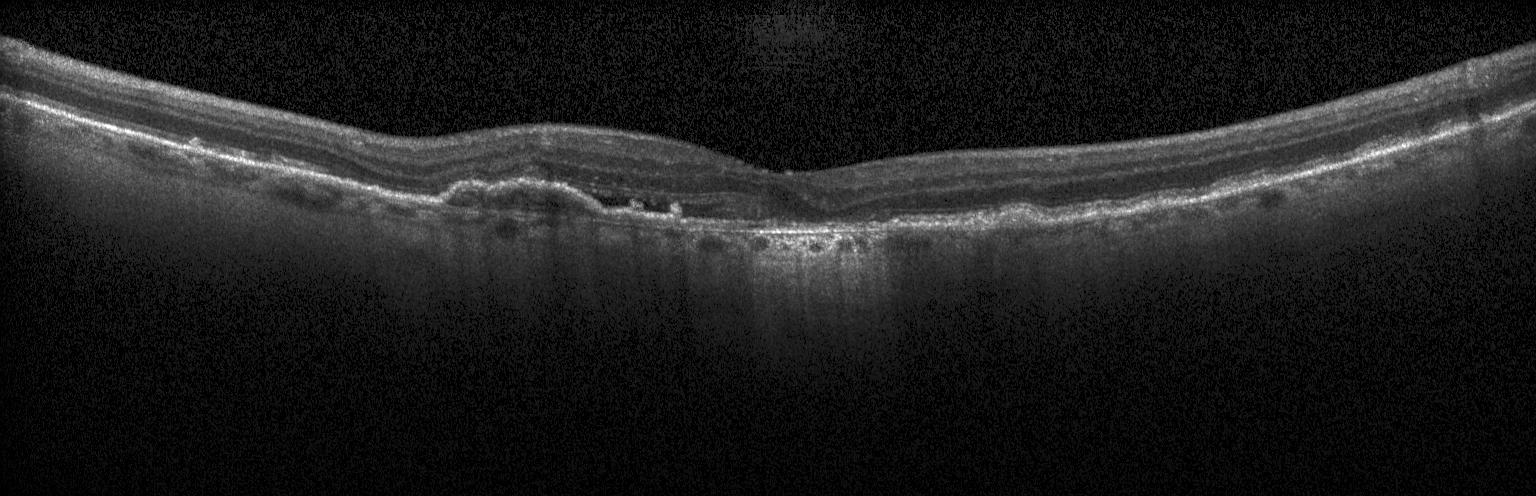 Diagnosis: a choroidal neovascular membrane.